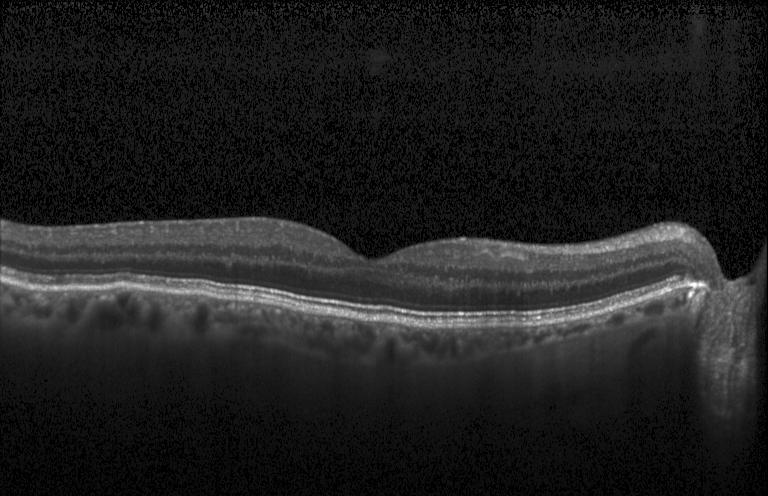
Assessment: no choroidal neovascularization, diabetic macular edema, or drusen.